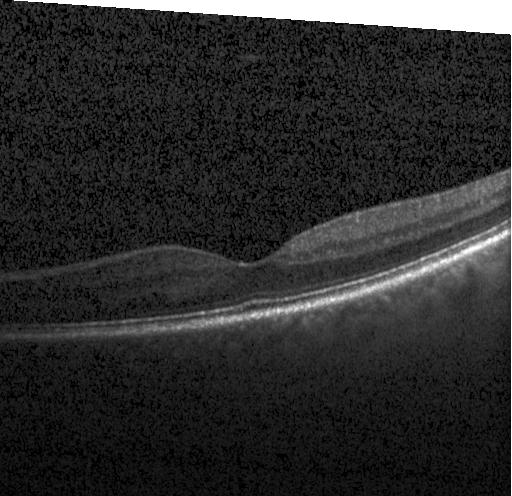

Macular OCT: neither choroidal neovascularization, diabetic macular edema, nor drusen.